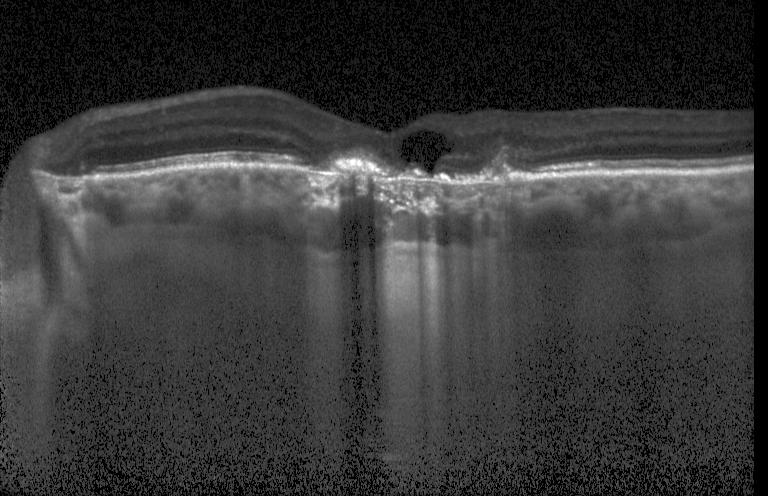

Retinal OCT cross-section.
OCT finding: choroidal neovascularization (CNV).